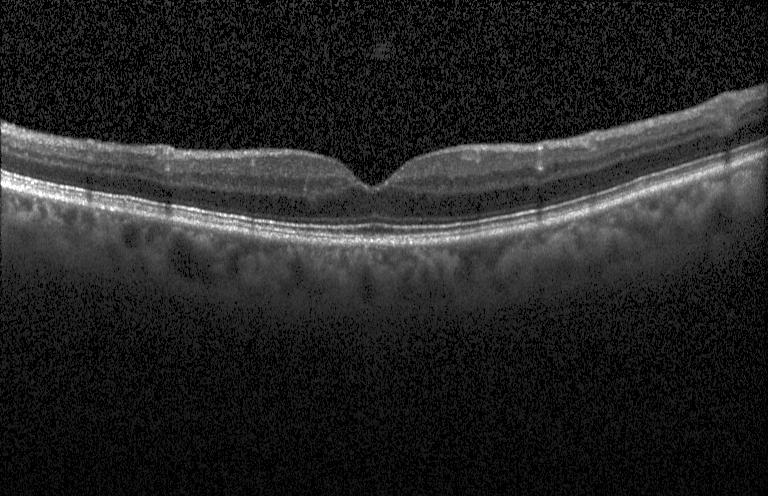

Acquired on a Heidelberg Spectralis; optical coherence tomography scan; SD-OCT — Macular OCT: no choroidal neovascularization, diabetic macular edema, or drusen.